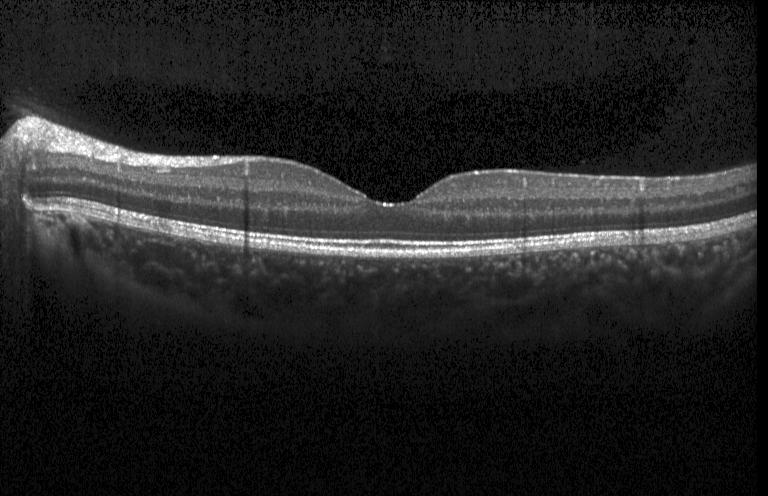
Macular scan. Optical coherence tomography B-scan. Acquired on a Heidelberg Spectralis. Spectral-domain OCT
OCT finding: no choroidal neovascularization, no diabetic macular edema, and no drusen.